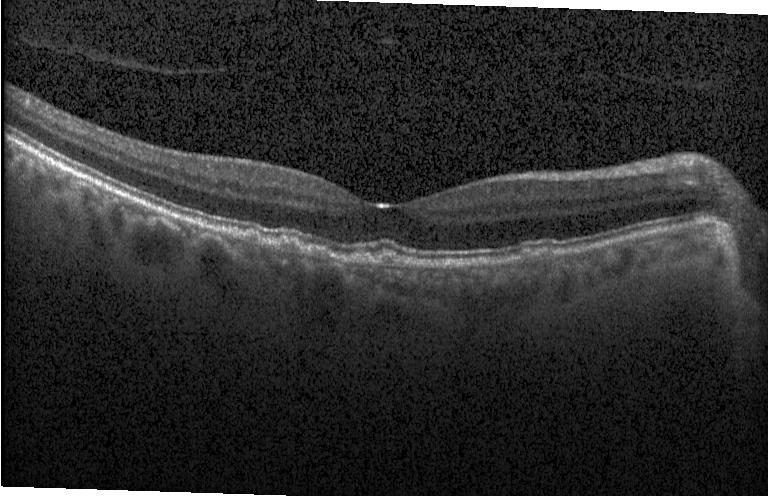
Heidelberg Spectralis OCT system. Retinal OCT cross-section
Multiple drusen.